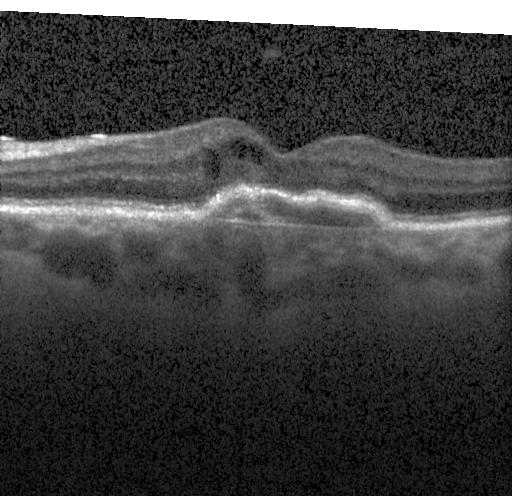 OCT B-scan; fovea-centered; Heidelberg Spectralis OCT system; spectral-domain optical coherence tomography. Diagnosis: a choroidal neovascular membrane.